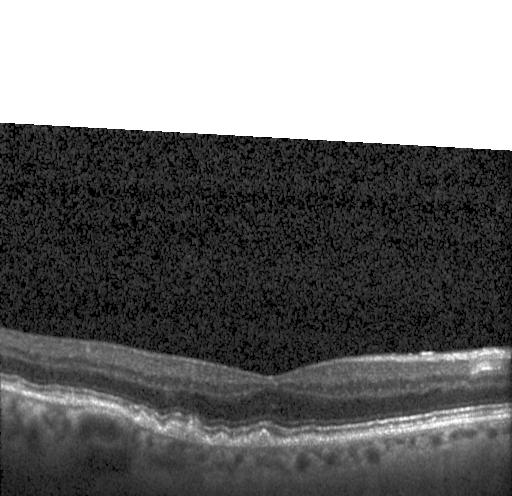 Spectral-domain OCT B-scan: sub-RPE drusenoid deposits.